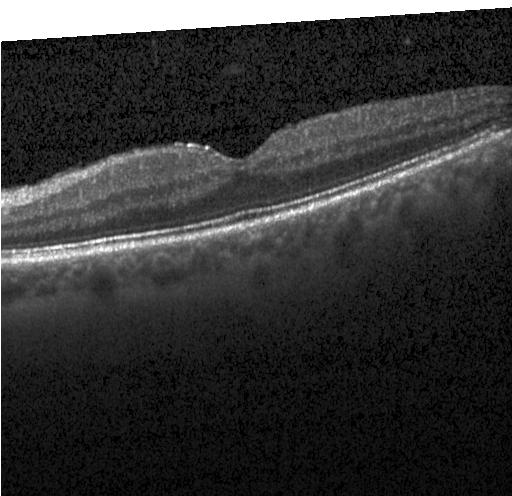 Retinal OCT cross-section · centered on the fovea · spectral-domain OCT · acquired on a Heidelberg Spectralis
No CNV, DME, or drusen.